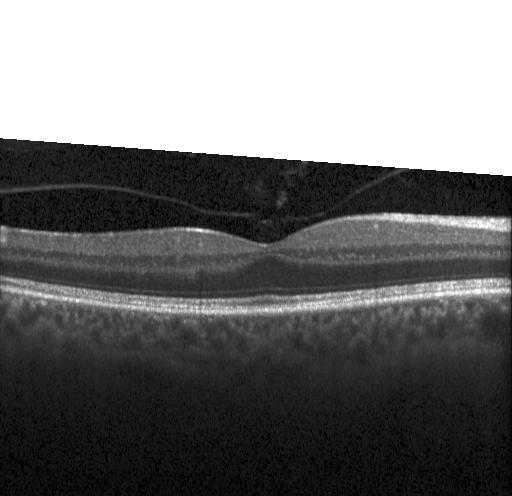 SD-OCT, acquired on a Heidelberg Spectralis, horizontal scan through the fovea, optical coherence tomography scan. Dx: no CNV, DME, or drusen.